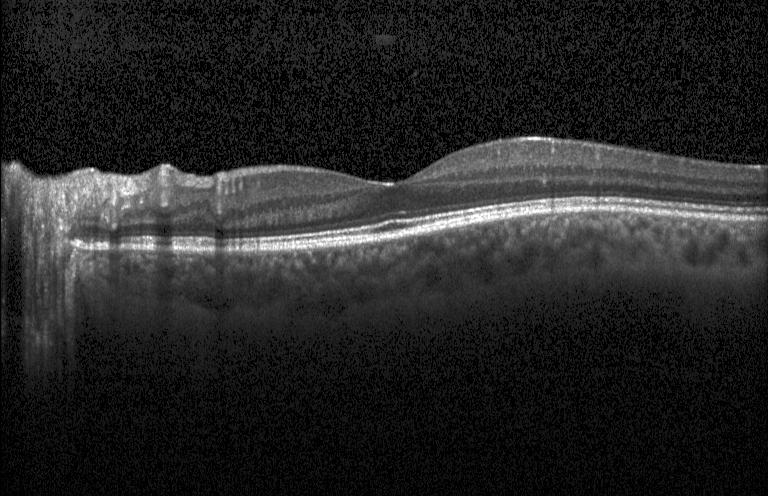
Heidelberg Spectralis OCT system. Retinal OCT cross-section. Spectral-domain OCT. Impression: no evidence of CNV, DME, or drusen.